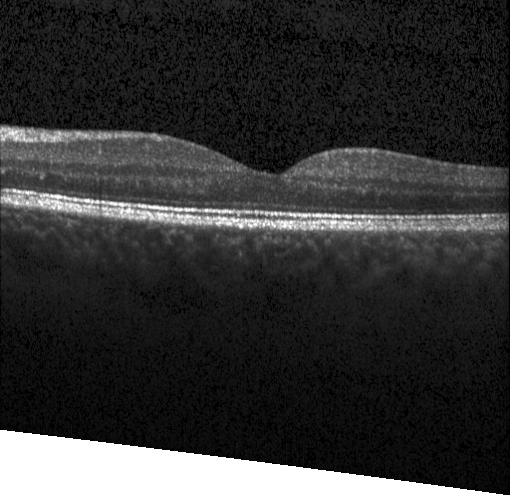

OCT B-scan showing no choroidal neovascularization, diabetic macular edema, or drusen.